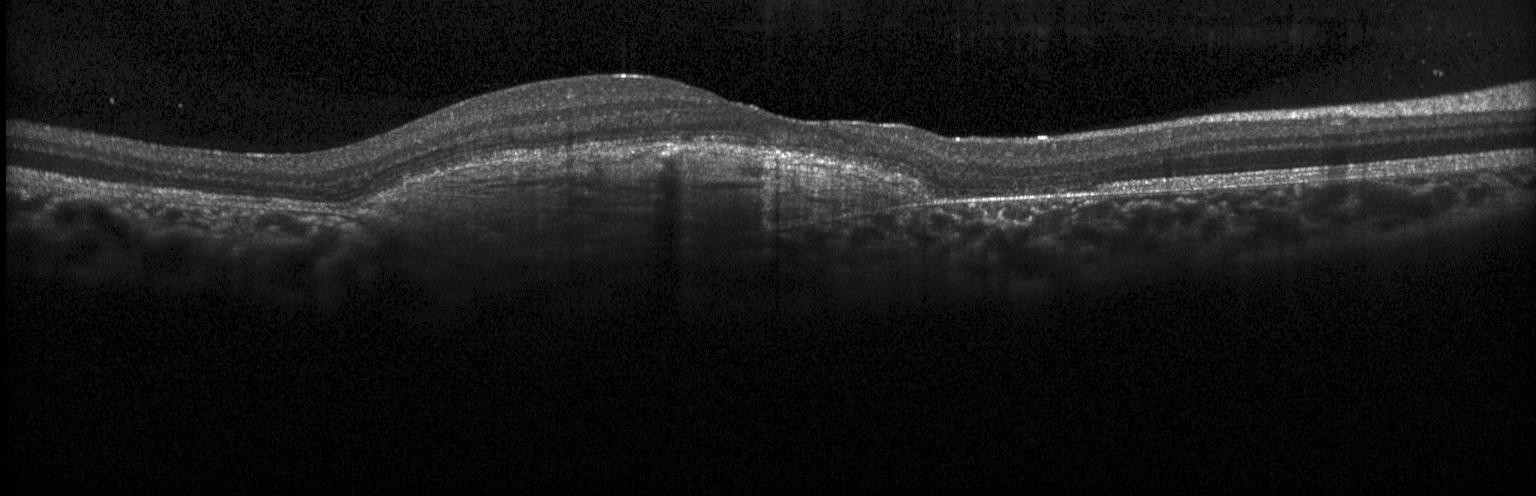
Assessment: choroidal neovascularization.